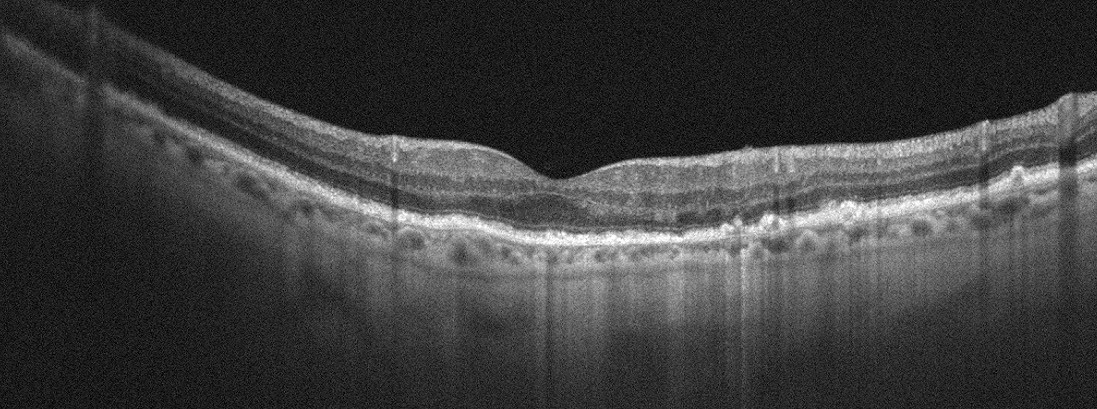

Dx: age-related macular degeneration.